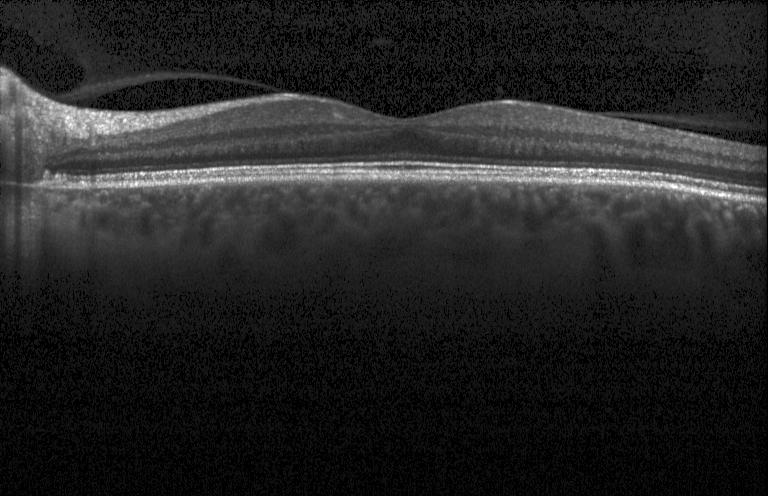

Retinal OCT B-scan.
Diagnosis: no choroidal neovascularization, no diabetic macular edema, and no drusen.